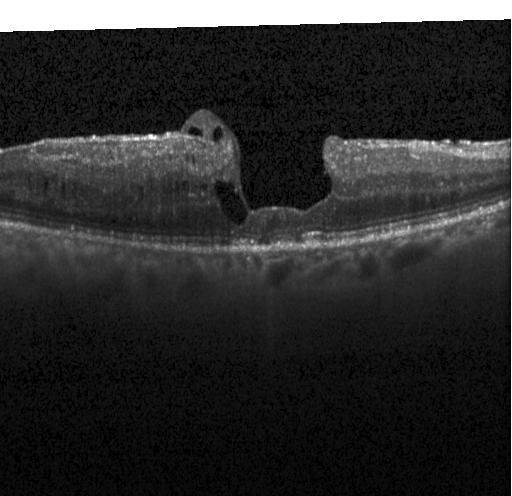 Impression: DME.